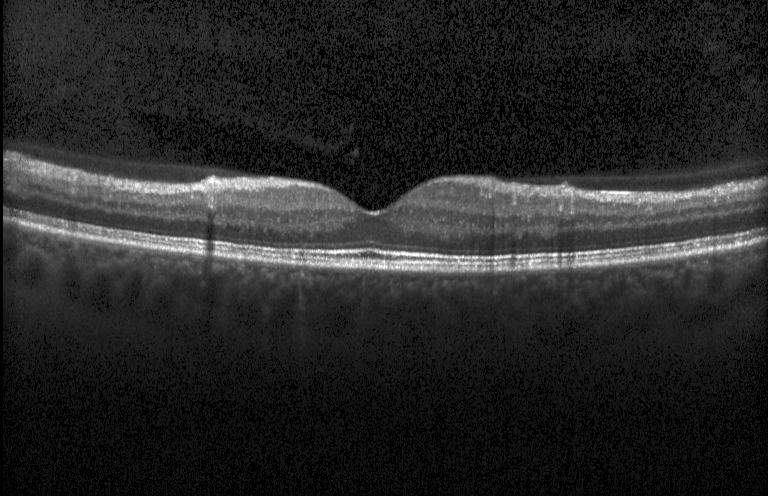

The scan shows no choroidal neovascularization, diabetic macular edema, or drusen.